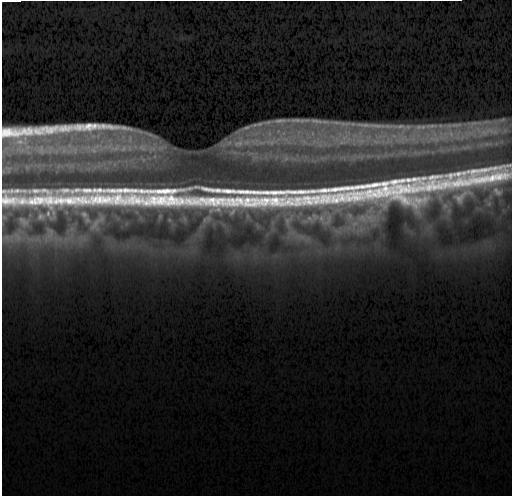
OCT finding: no evidence of CNV, DME, or drusen.